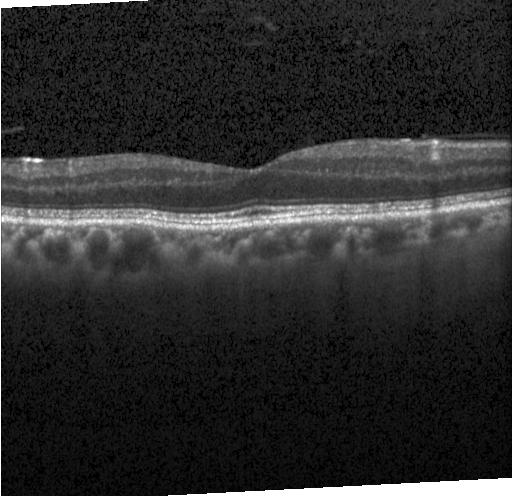

Optical coherence tomography scan · spectral-domain optical coherence tomography
OCT finding: no choroidal neovascularization, diabetic macular edema, or drusen.